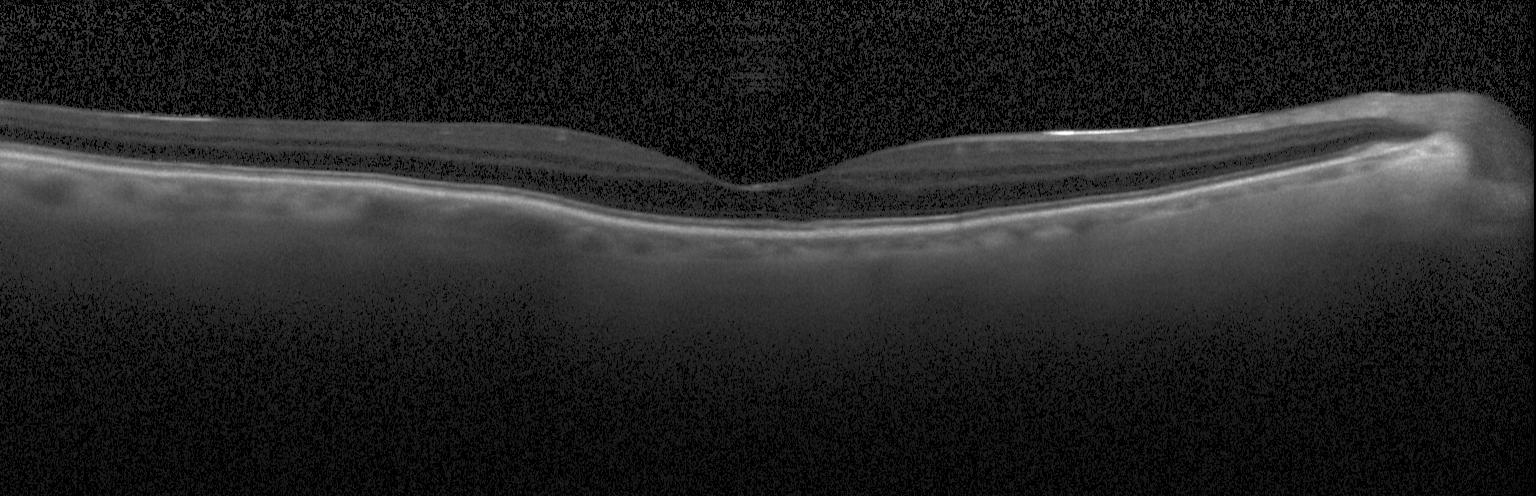 Heidelberg Spectralis · retinal OCT cross-section · horizontal scan through the fovea
Assessment: no CNV, DME, or drusen.